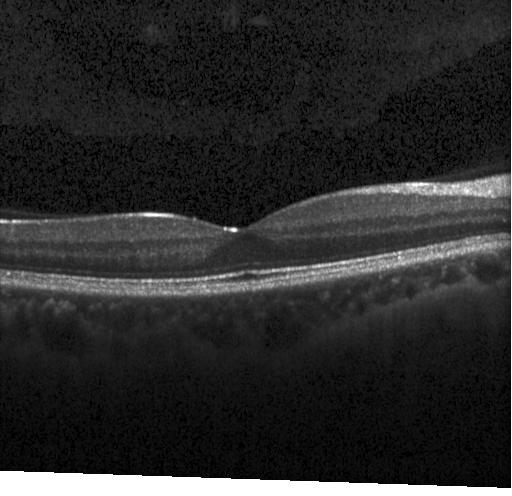
Macular OCT: no choroidal neovascularization, no diabetic macular edema, and no drusen.